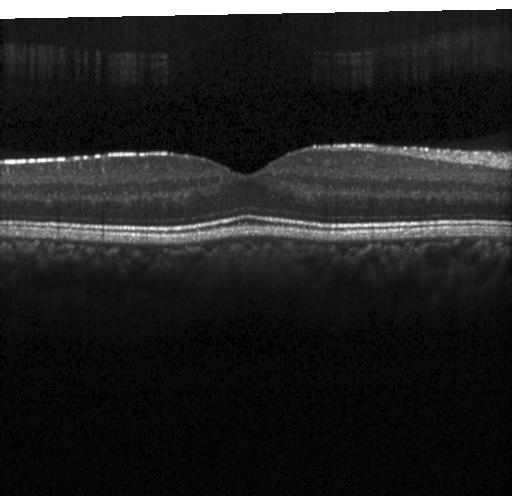 Heidelberg Spectralis OCT system. Fovea-centered. Spectral-domain OCT. Optical coherence tomography B-scan.
Dx: no choroidal neovascularization, diabetic macular edema, or drusen.